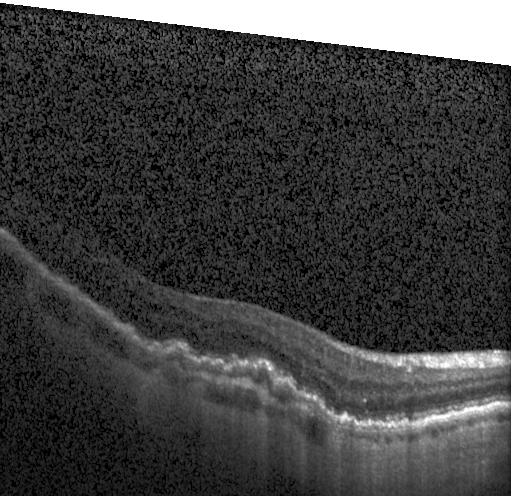 Macular OCT demonstrating a choroidal neovascular membrane.